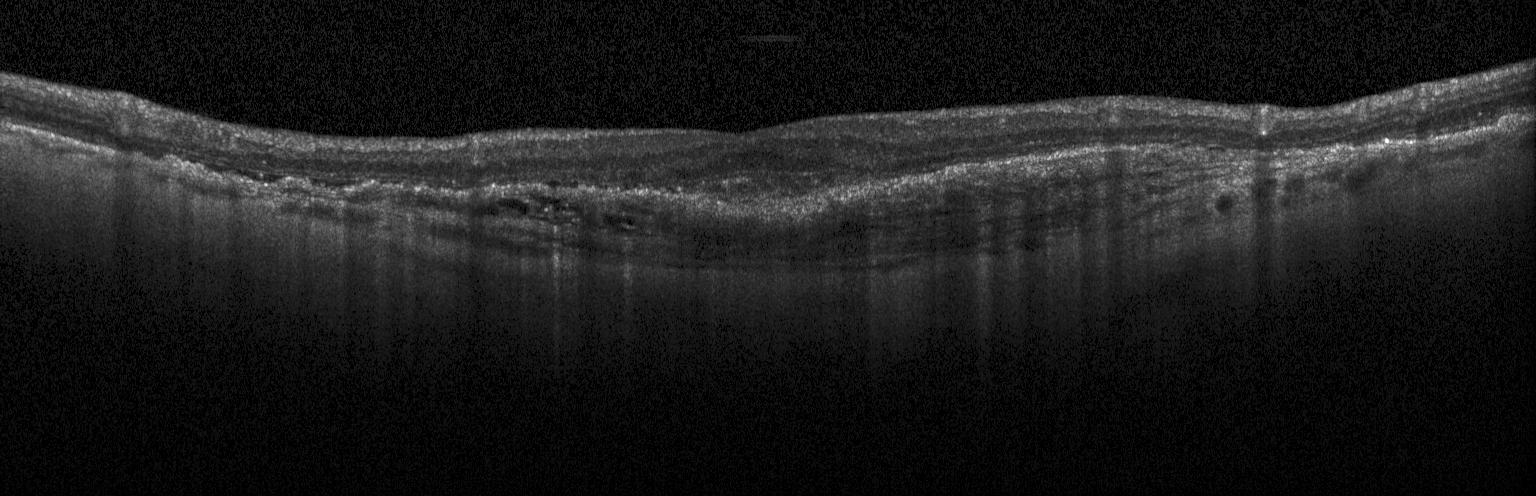

Macular OCT: choroidal neovascularization (CNV).